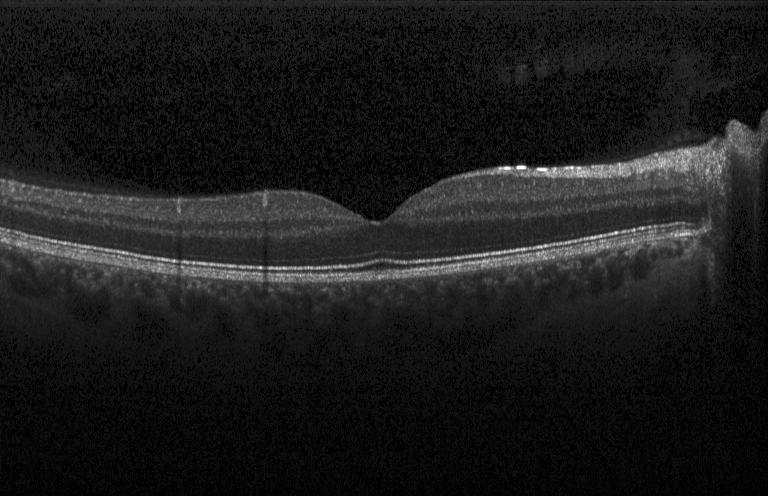

Finding: no choroidal neovascularization, diabetic macular edema, or drusen.